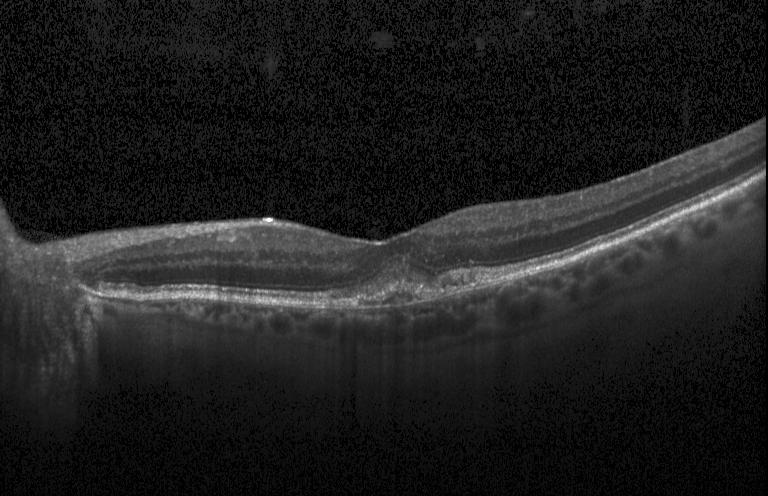 OCT scan showing choroidal neovascularization.